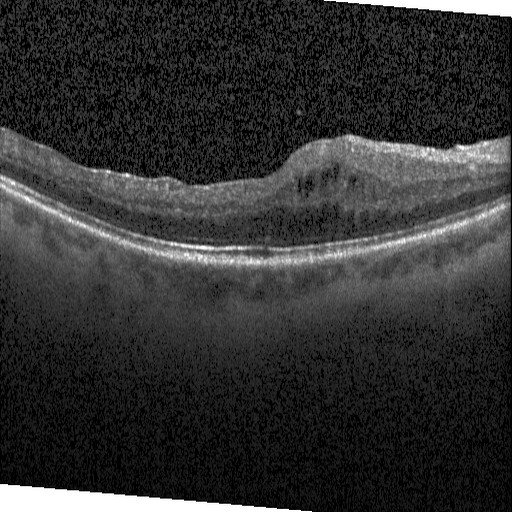

Diagnosis: diabetic macular edema (DME).